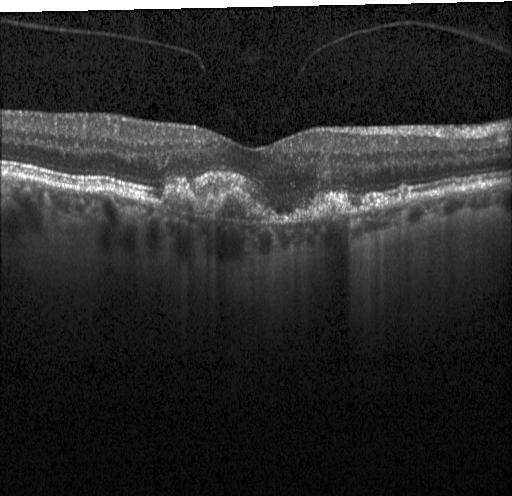

Through the macula; OCT line scan.
Finding: choroidal neovascularization (CNV).